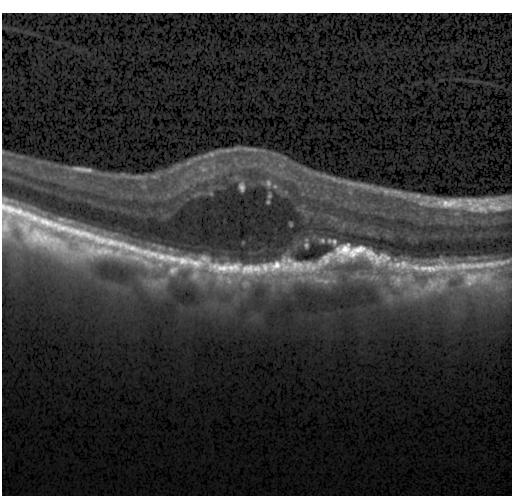 Impression: a choroidal neovascular membrane.